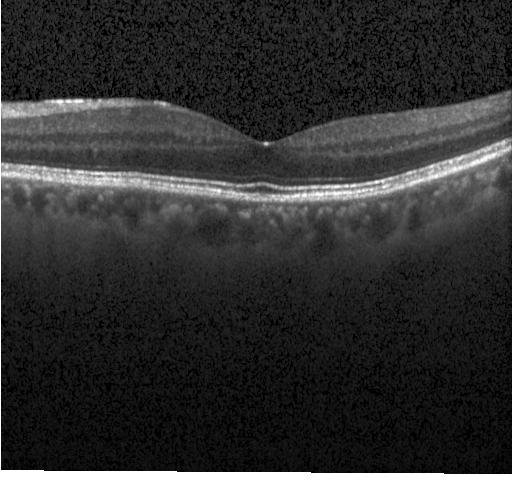
Retinal OCT cross-section · SD-OCT — Assessment: no evidence of choroidal neovascularization, diabetic macular edema, or drusen.